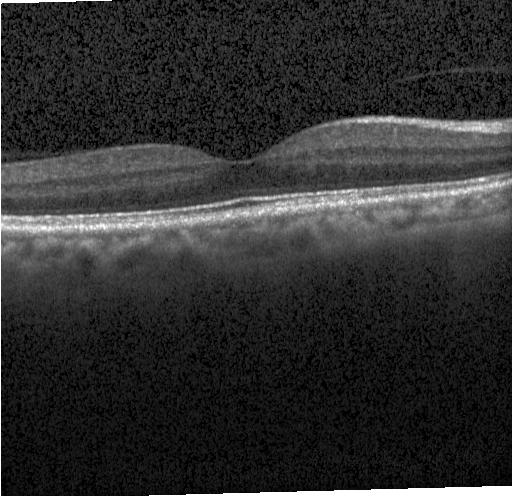 Macular OCT: no choroidal neovascularization, diabetic macular edema, or drusen.